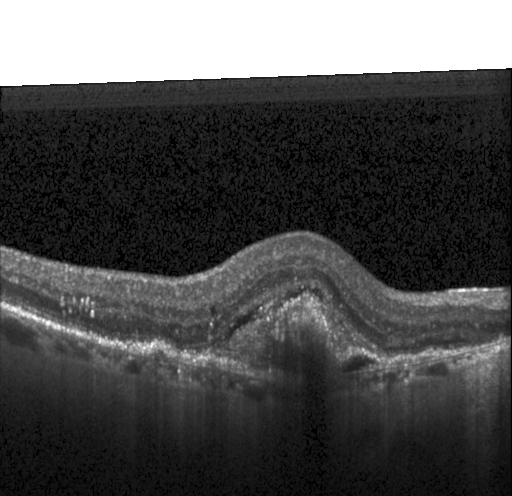

Retinal OCT cross-section — Macular OCT: choroidal neovascularization (CNV).